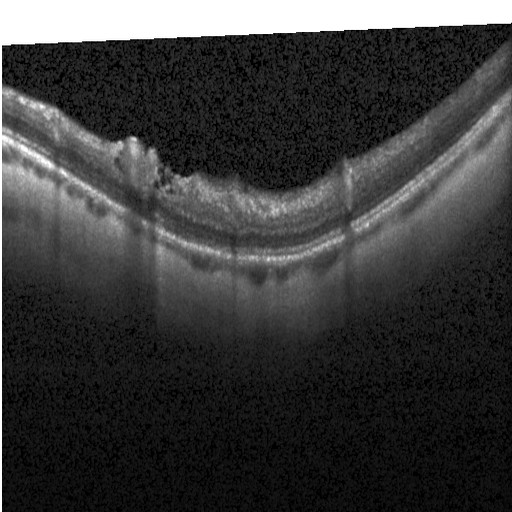

Acquired on a Heidelberg Spectralis, optical coherence tomography scan, through the macula, spectral-domain OCT. Impression: diabetic macular edema.